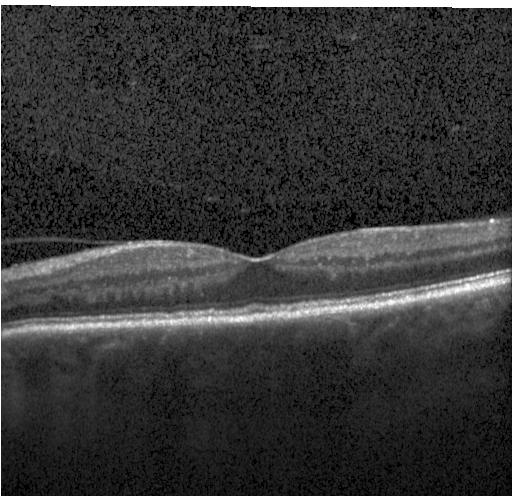

Spectral-domain OCT B-scan: no evidence of CNV, DME, or drusen.